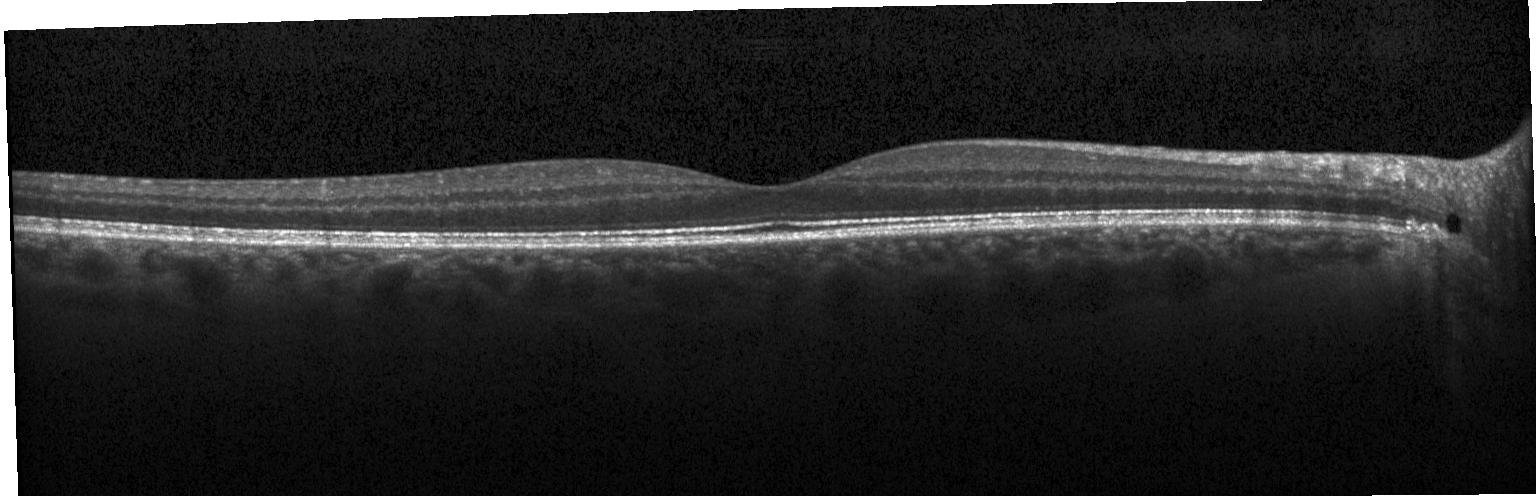

Retinal OCT B-scan
Finding: no choroidal neovascularization, no diabetic macular edema, and no drusen.